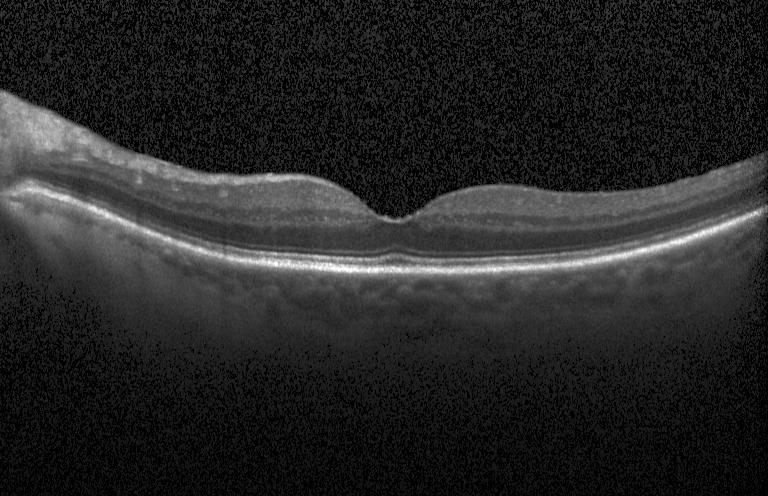 Horizontal scan through the fovea. Heidelberg Spectralis. Spectral-domain optical coherence tomography. Retinal OCT B-scan.
Impression: no choroidal neovascularization, diabetic macular edema, or drusen.